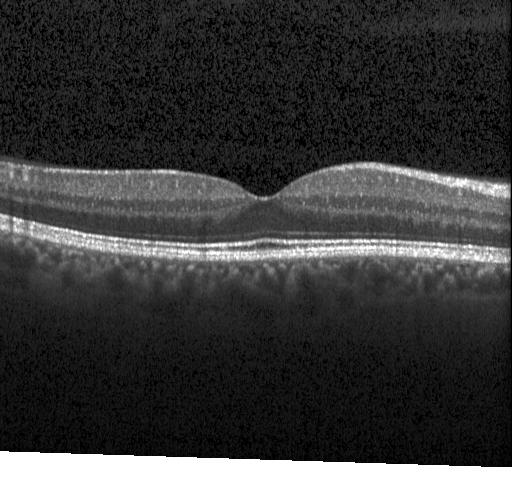

Spectral-domain OCT B-scan: no choroidal neovascularization, diabetic macular edema, or drusen.